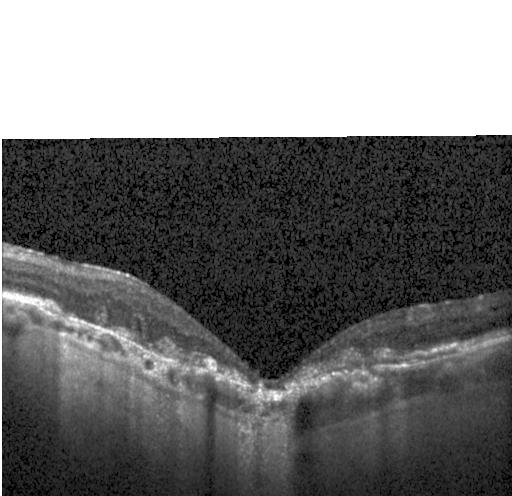
Retinal OCT cross-section.
Impression: choroidal neovascularization (CNV).